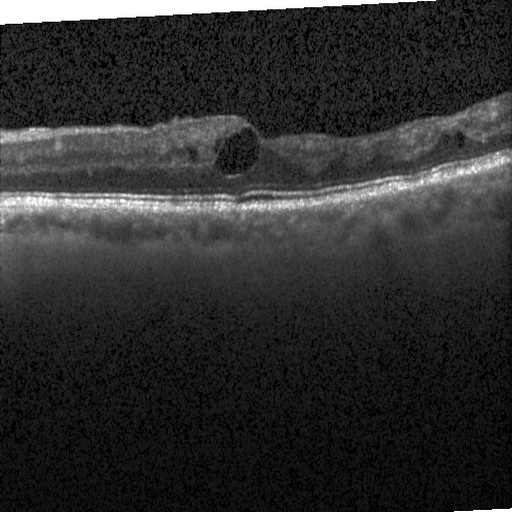

Retinal OCT B-scan — Diagnosis: DME.